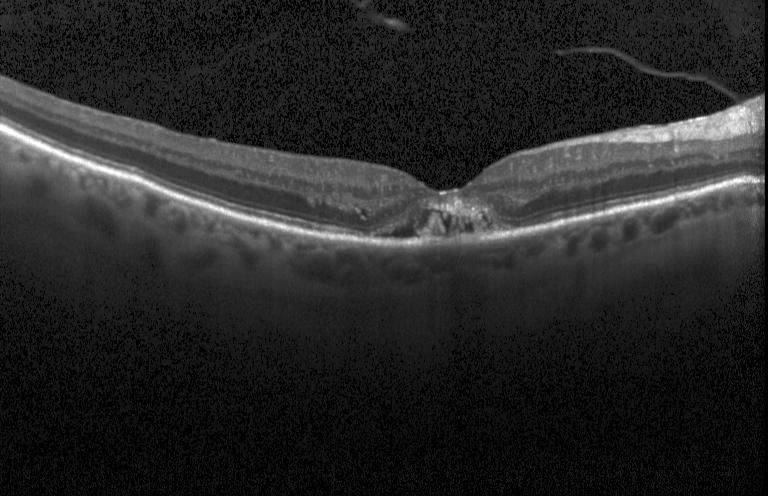

Acquired on a Heidelberg Spectralis. Retinal OCT cross-section. Diagnosis: choroidal neovascularization (CNV).